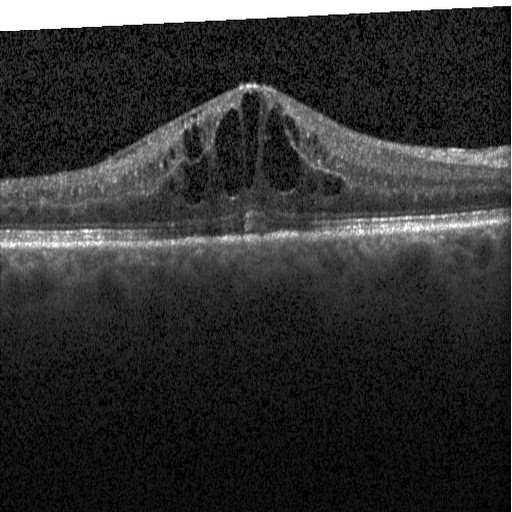 Diabetic macular edema (DME).